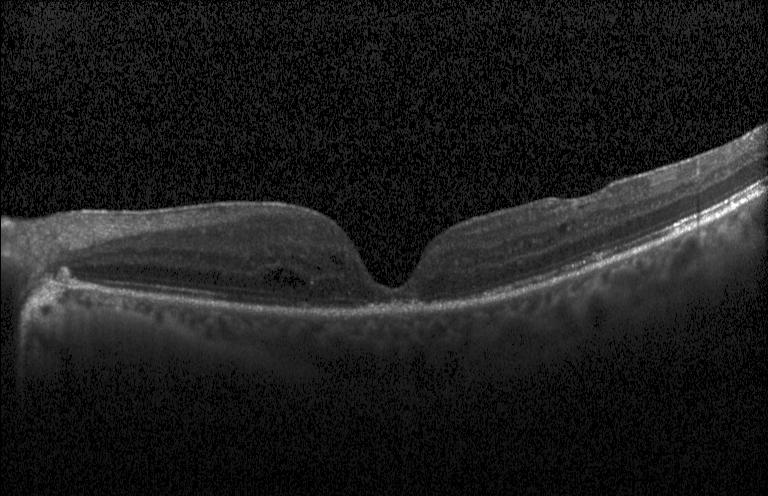

OCT scan showing diabetic macular edema (DME).